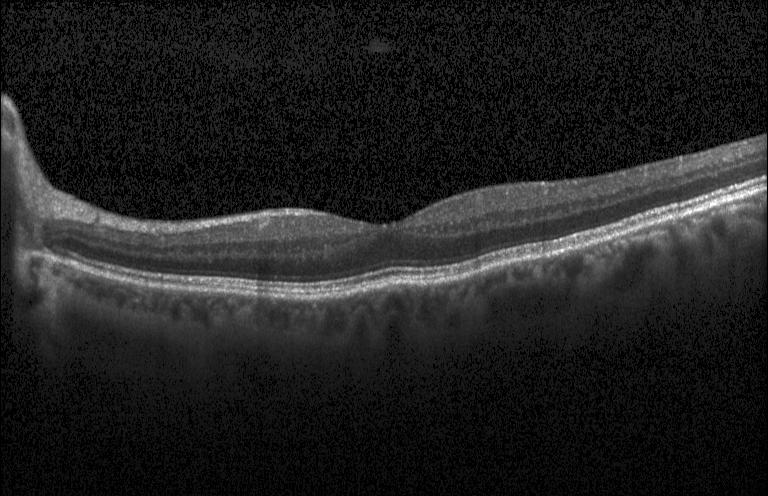 Heidelberg Spectralis; optical coherence tomography scan. Diagnosis: no evidence of CNV, DME, or drusen.